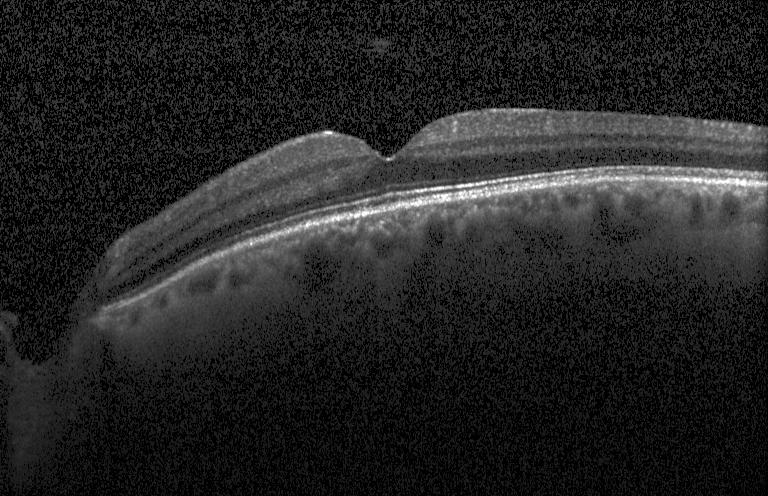

Macular OCT: neither choroidal neovascularization, diabetic macular edema, nor drusen.